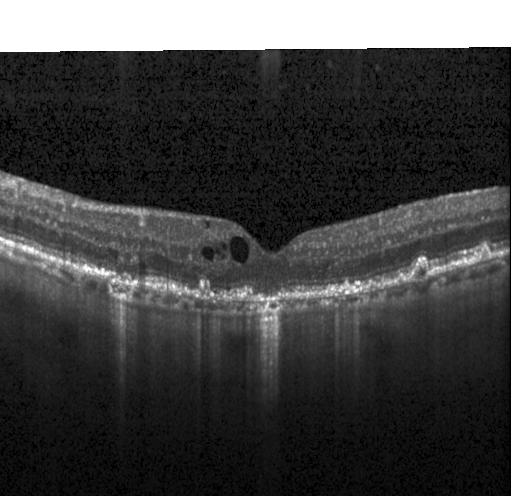

OCT B-scan showing CNV.